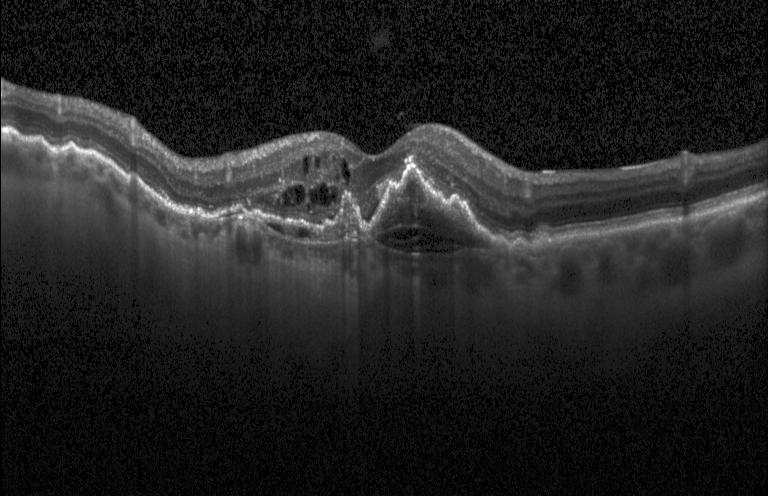
OCT line scan — Dx: CNV.